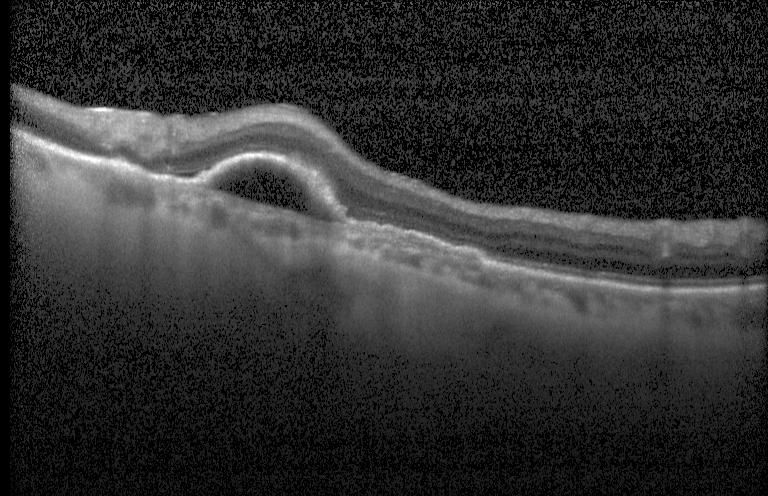

OCT B-scan showing choroidal neovascularization.